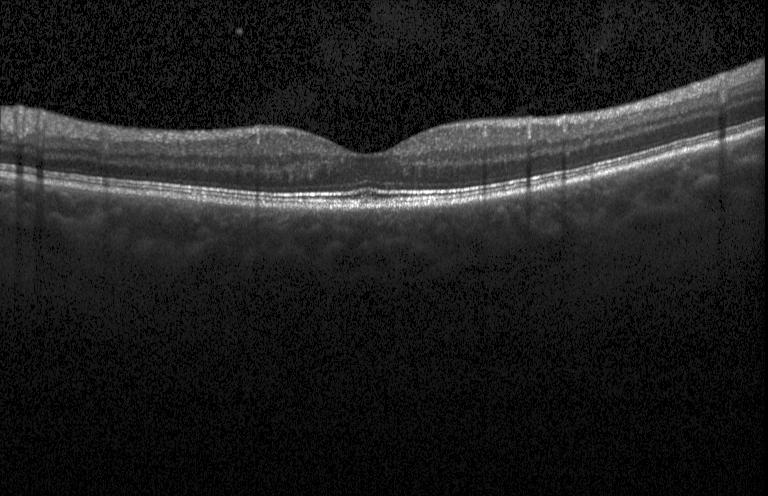
OCT scan showing neither choroidal neovascularization, diabetic macular edema, nor drusen.